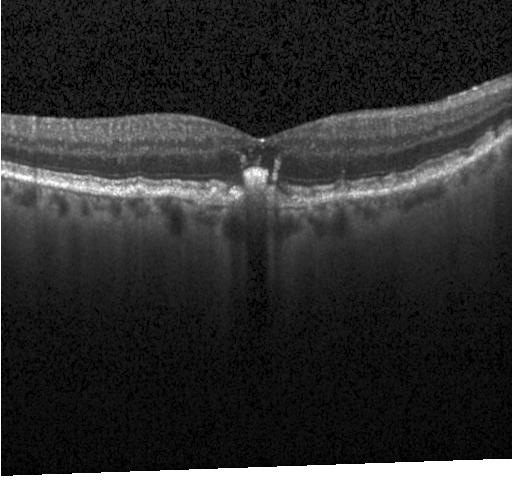

OCT finding: drusen.